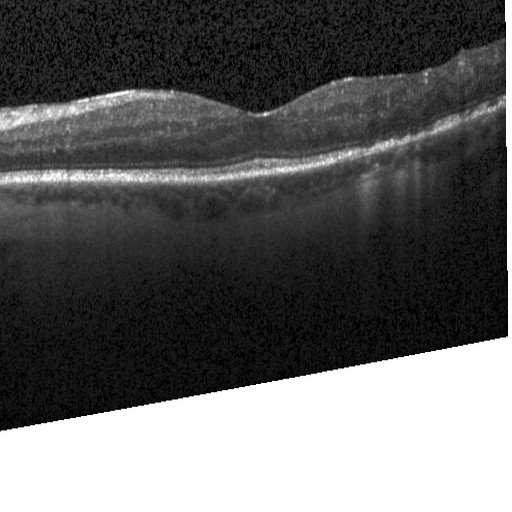
Optical coherence tomography B-scan · instrument: Heidelberg Spectralis · SD-OCT · through the macula — Diagnosis: DME.